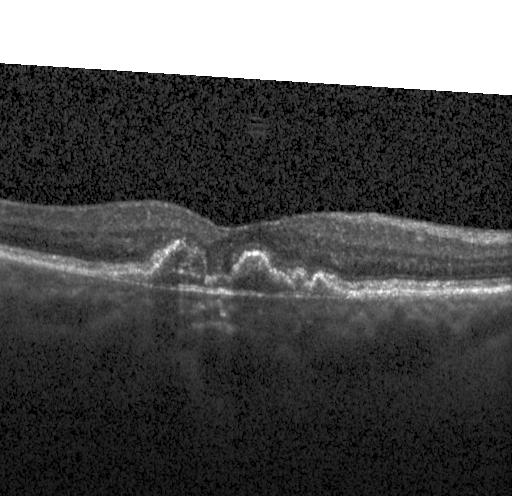

Through the macula · instrument: Heidelberg Spectralis · spectral-domain OCT · OCT B-scan.
The scan shows a choroidal neovascular membrane.